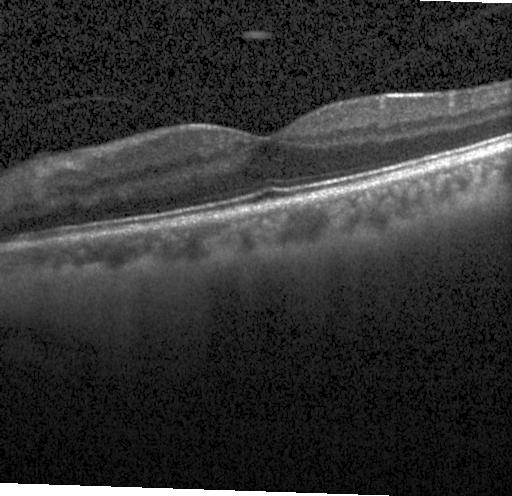
Spectral-domain optical coherence tomography, acquired on a Heidelberg Spectralis, centered on the fovea, retinal OCT B-scan — Neither CNV, DME, nor drusen.